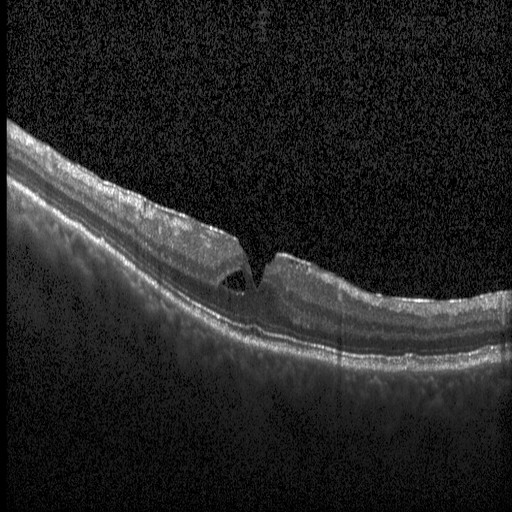

Centered on the fovea · optical coherence tomography B-scan · Heidelberg Spectralis OCT system · SD-OCT. Assessment: diabetic macular edema.